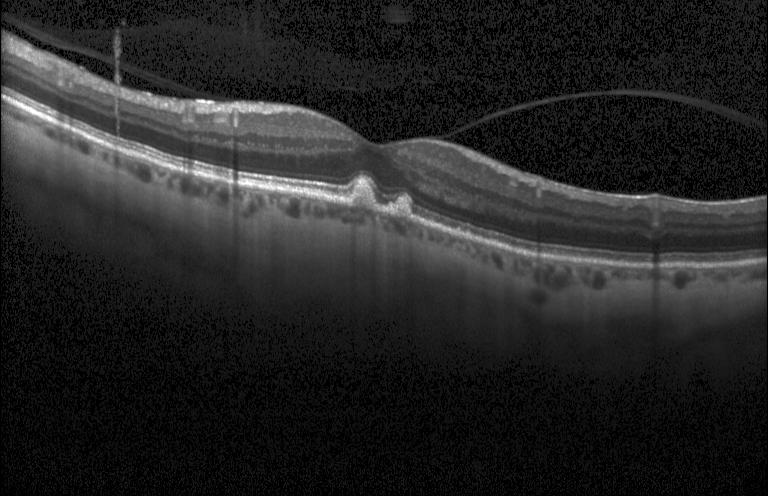

Optical coherence tomography B-scan. Fovea-centered. Spectral-domain OCT.
Finding: drusen.